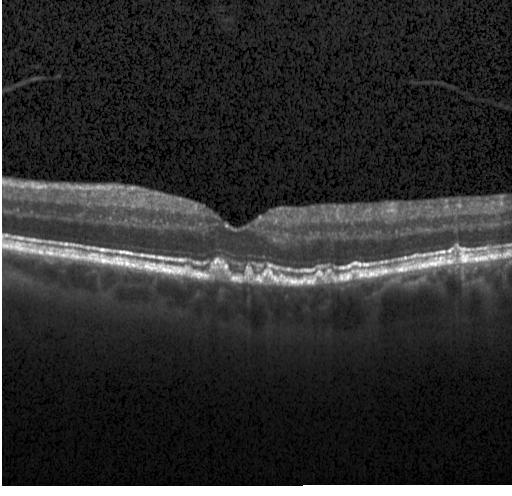

Diagnosis: sub-RPE drusenoid deposits.